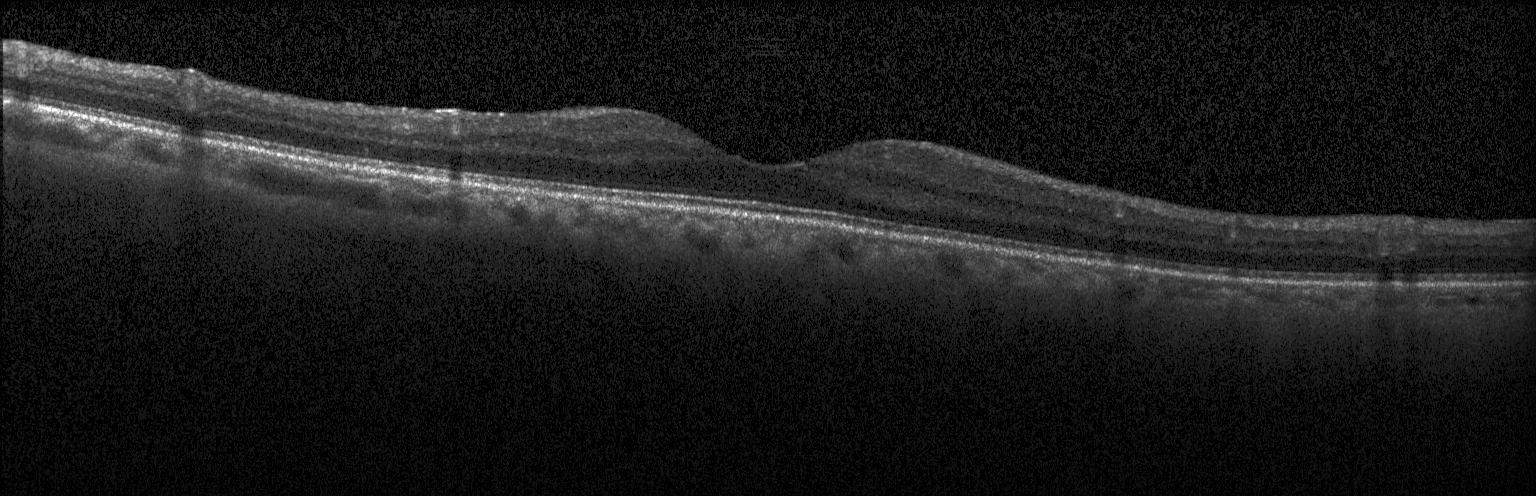
Diagnosis: neither choroidal neovascularization, diabetic macular edema, nor drusen.